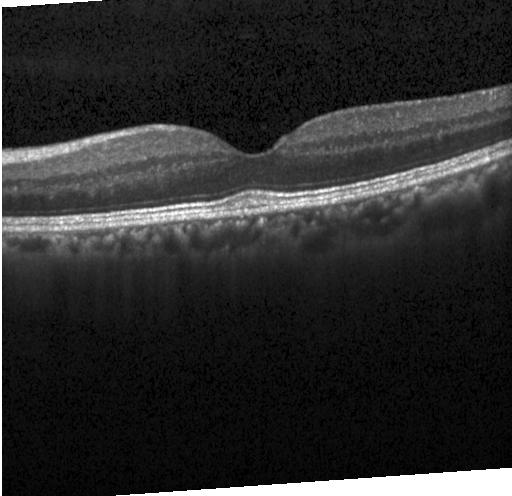
Optical coherence tomography B-scan.
Macular OCT: no evidence of choroidal neovascularization, diabetic macular edema, or drusen.